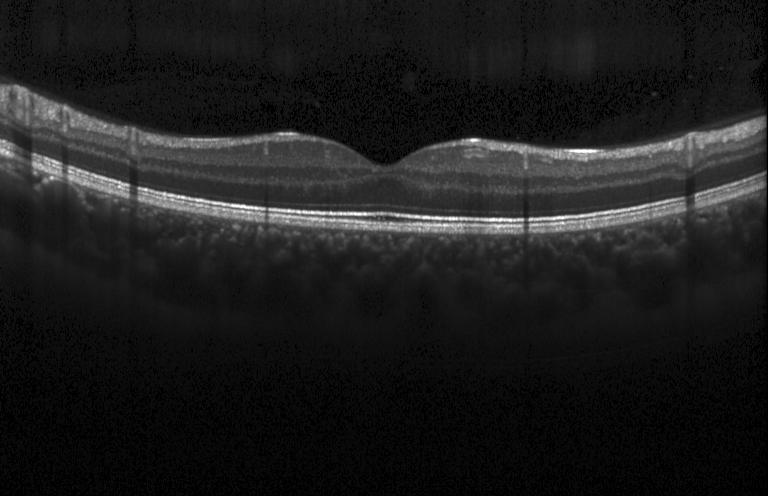 OCT B-scan; fovea-centered — This B-scan demonstrates no CNV, DME, or drusen.